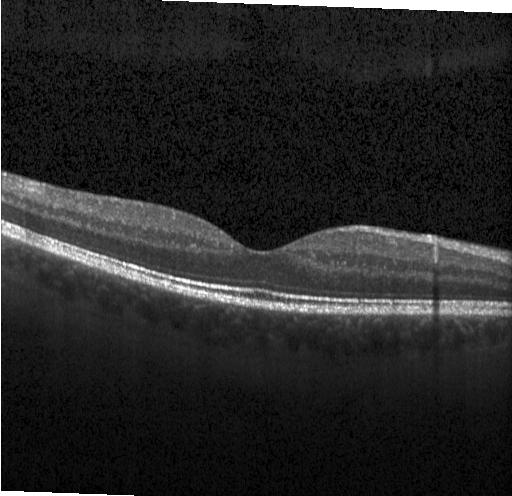
Macular OCT: no choroidal neovascularization, diabetic macular edema, or drusen.